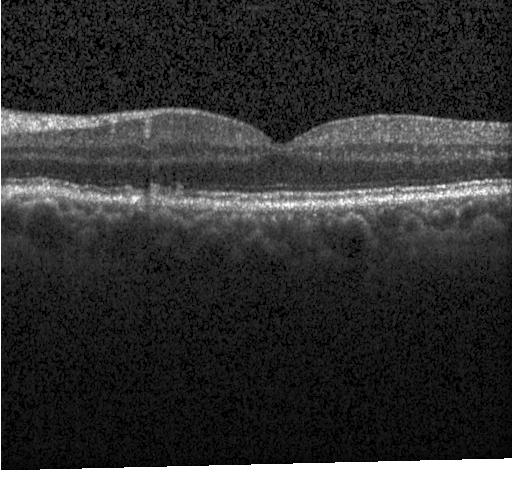

Finding: multiple drusen.